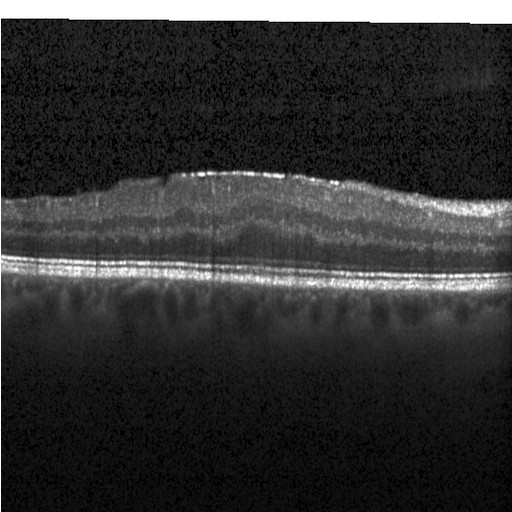

OCT B-scan showing diabetic macular edema.